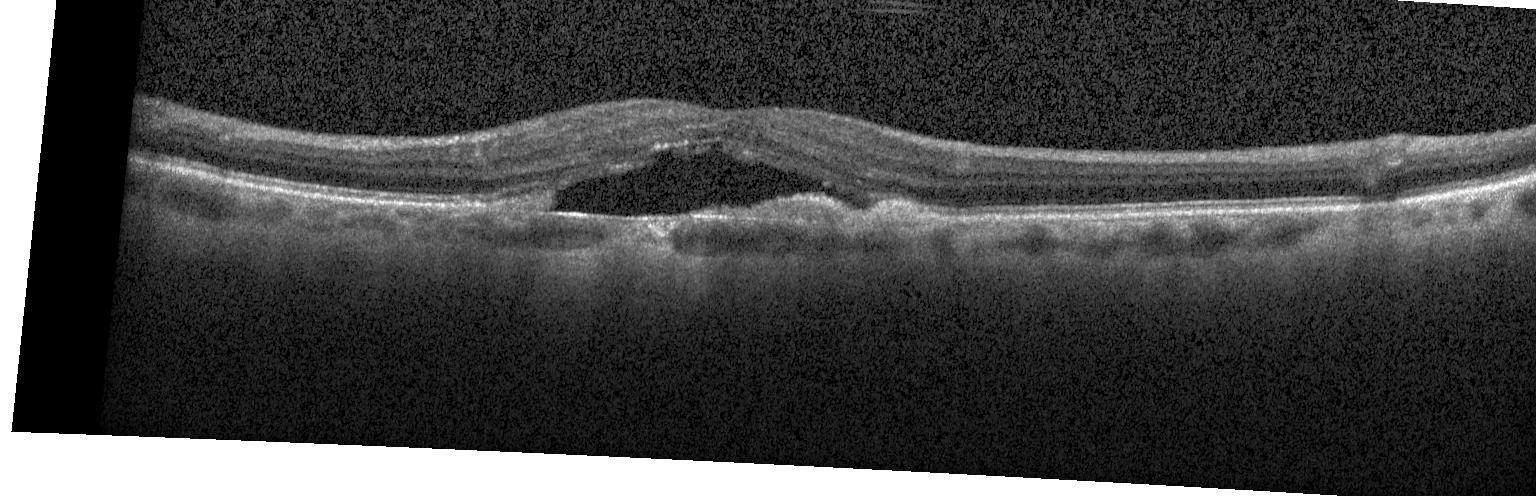
Spectral-domain optical coherence tomography; Heidelberg Spectralis OCT system; retinal OCT B-scan.
OCT finding: CNV.